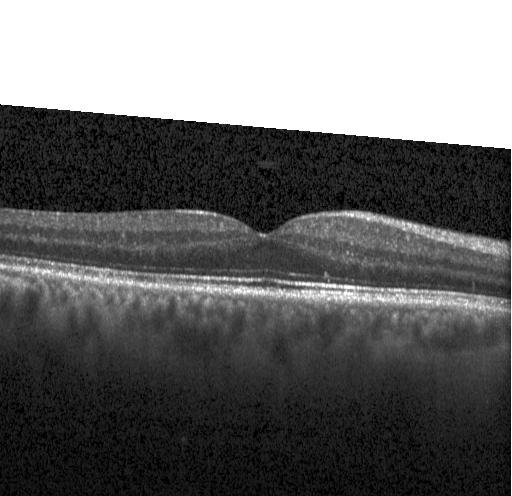 Neither choroidal neovascularization, diabetic macular edema, nor drusen.